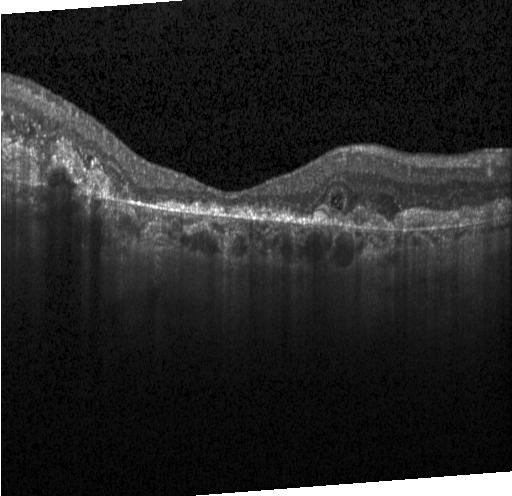

OCT B-scan · macular scan
Impression: a choroidal neovascular membrane.